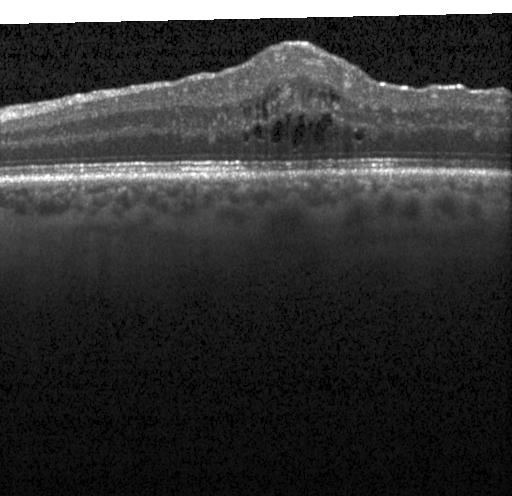 Retinal OCT cross-section showing diabetic macular edema (DME).